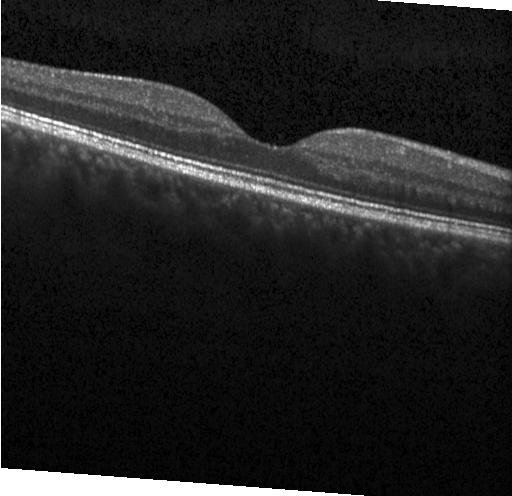 Diagnosis: no choroidal neovascularization, no diabetic macular edema, and no drusen.